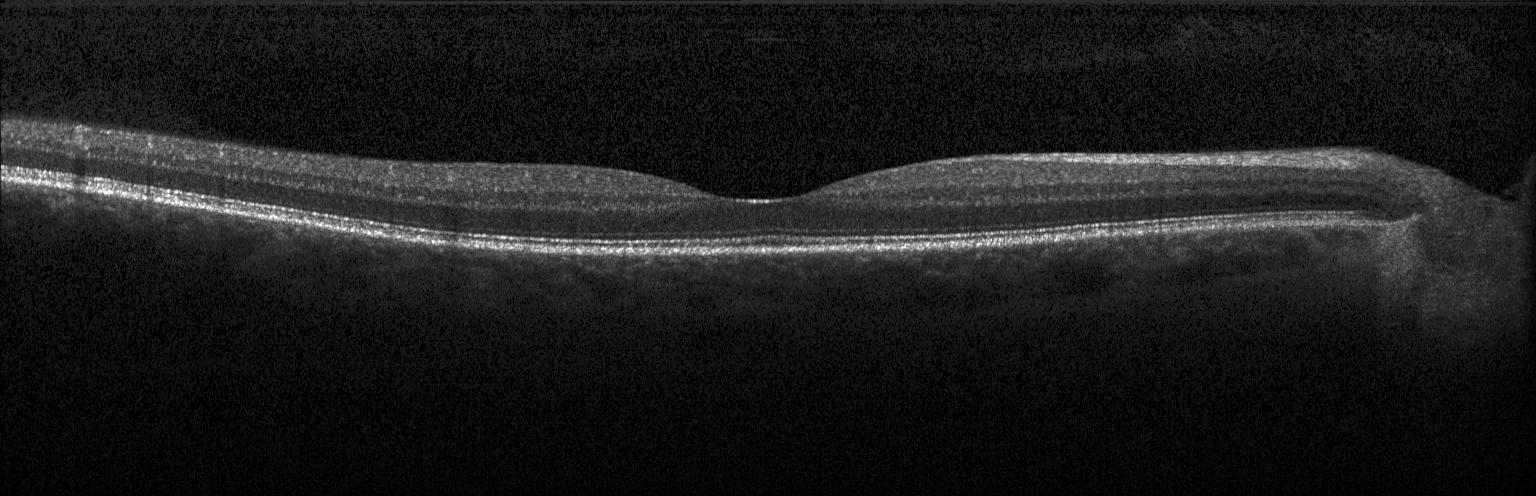
Spectral-domain optical coherence tomography; retinal OCT cross-section; fovea-centered; acquired on a Heidelberg Spectralis — Diagnosis: no CNV, no DME, and no drusen.